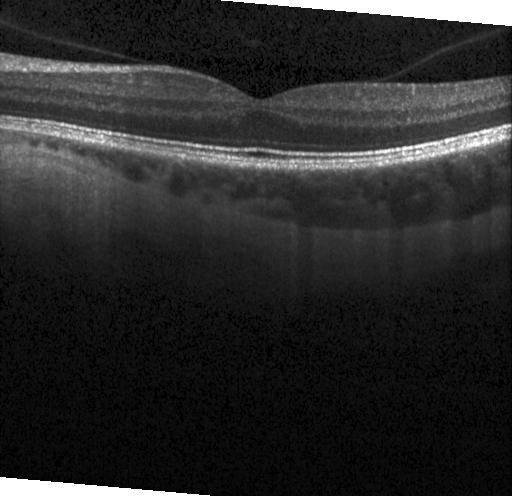
Diagnosis: no CNV, DME, or drusen.